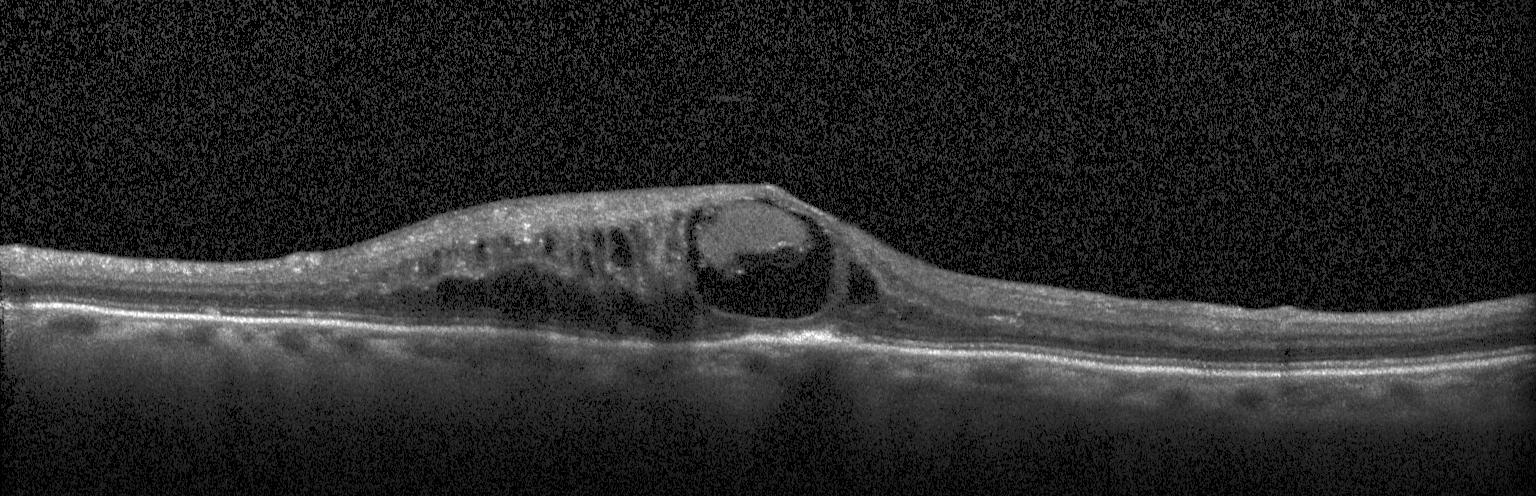
Optical coherence tomography B-scan · through the macula — Finding: diabetic macular edema (DME).